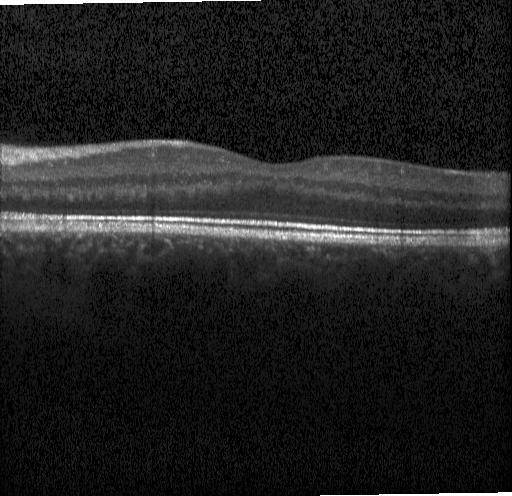 Optical coherence tomography scan · Heidelberg Spectralis · SD-OCT
The scan shows no choroidal neovascularization, no diabetic macular edema, and no drusen.